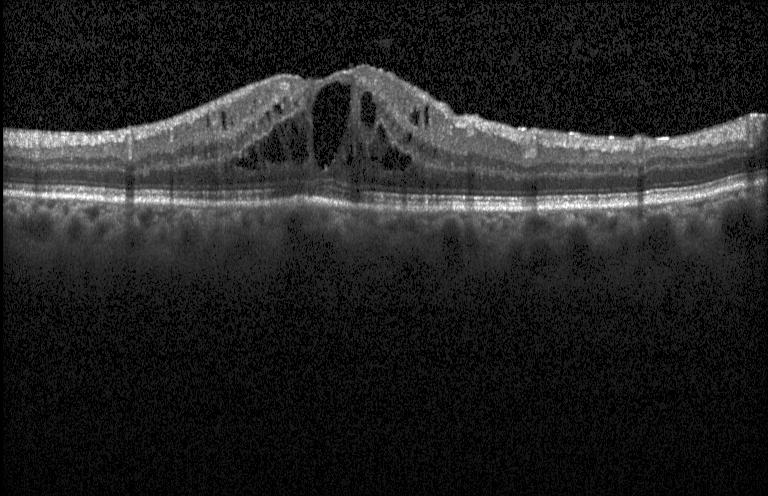

SD-OCT. Retinal OCT B-scan.
Impression: diabetic macular edema.